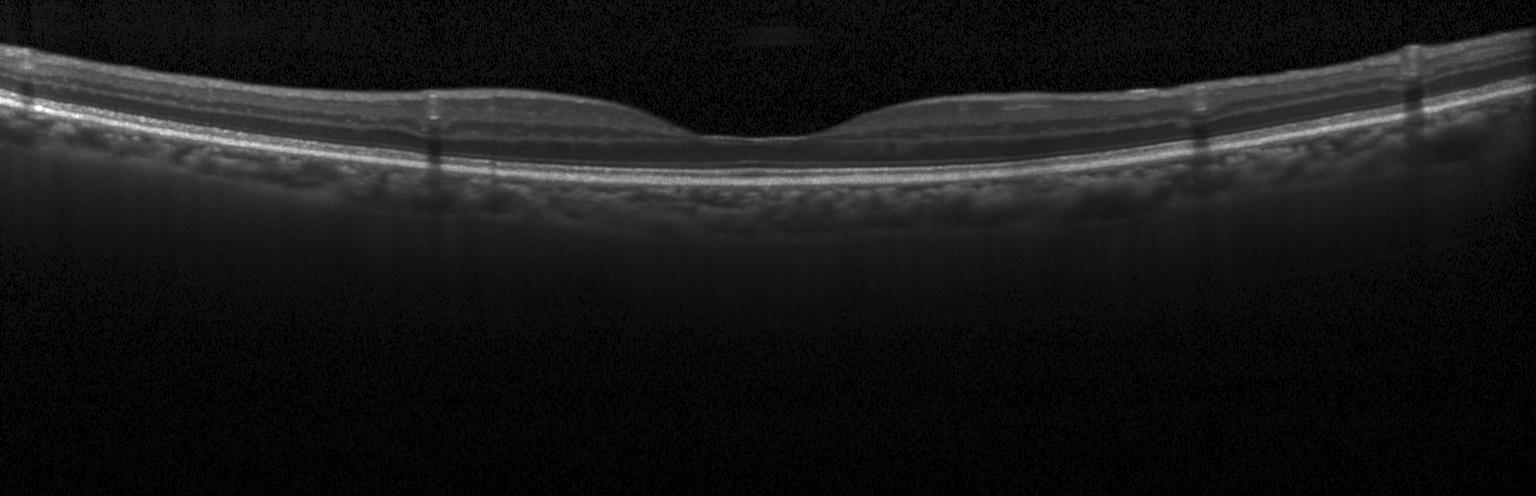 Spectral-domain optical coherence tomography; optical coherence tomography scan.
No evidence of choroidal neovascularization, diabetic macular edema, or drusen.